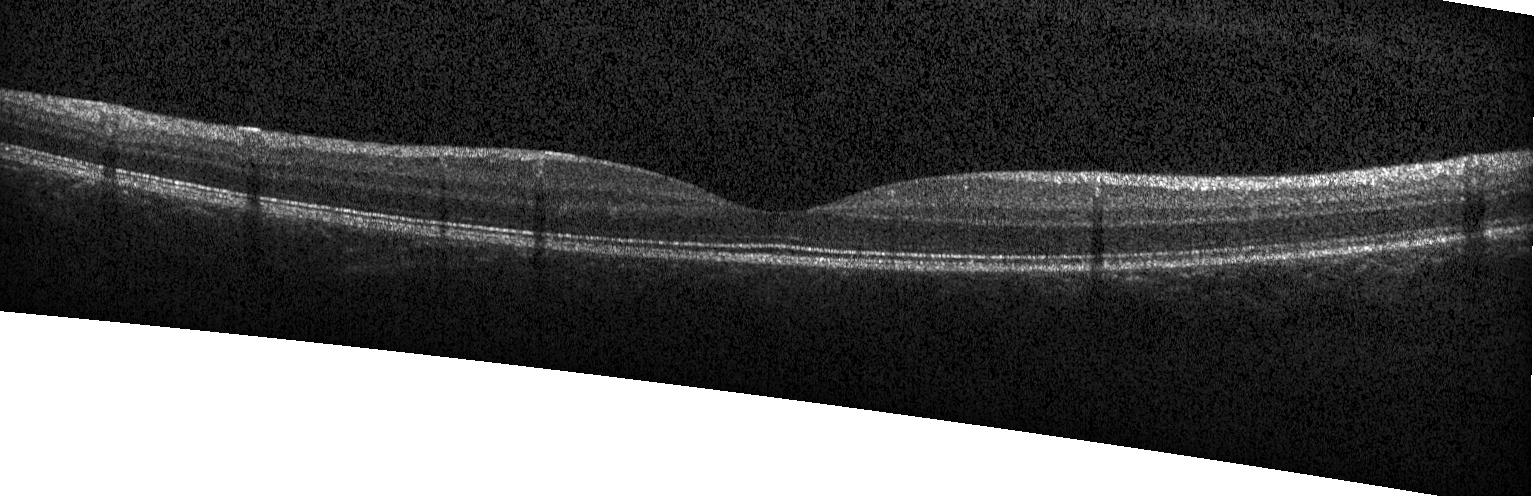
Heidelberg Spectralis · OCT line scan
Impression: no evidence of choroidal neovascularization, diabetic macular edema, or drusen.